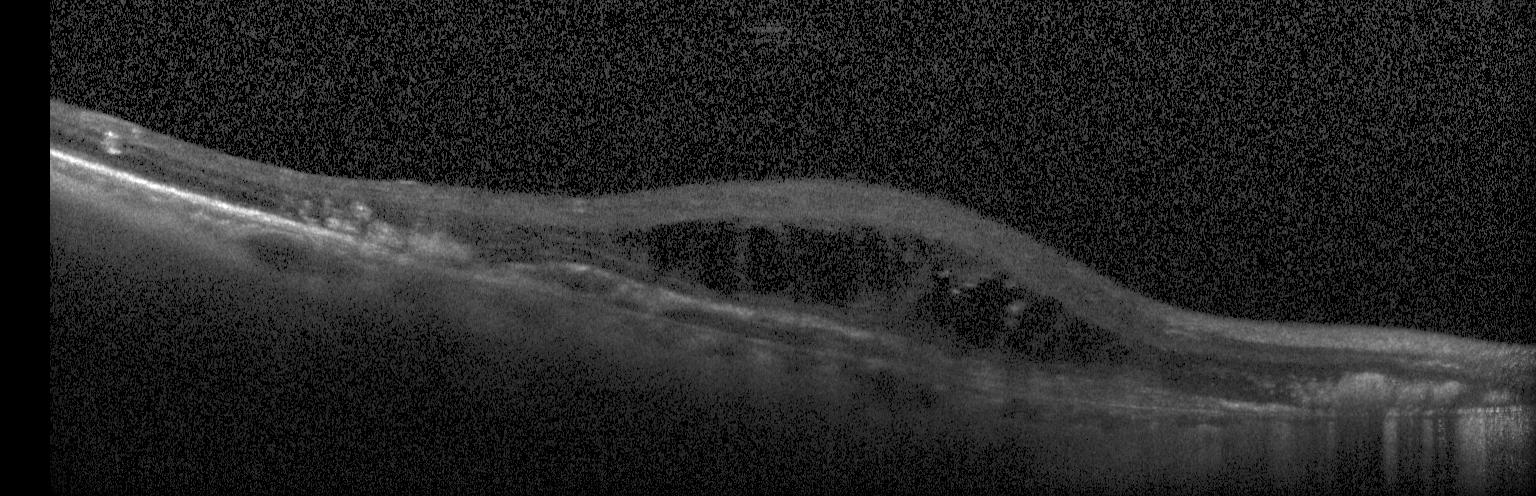 Retinal OCT B-scan. Heidelberg Spectralis. Fovea-centered. SD-OCT
This B-scan demonstrates a choroidal neovascular membrane.